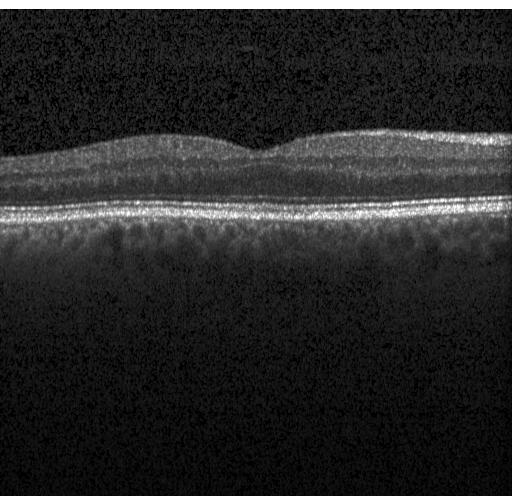 Diagnosis: neither choroidal neovascularization, diabetic macular edema, nor drusen.